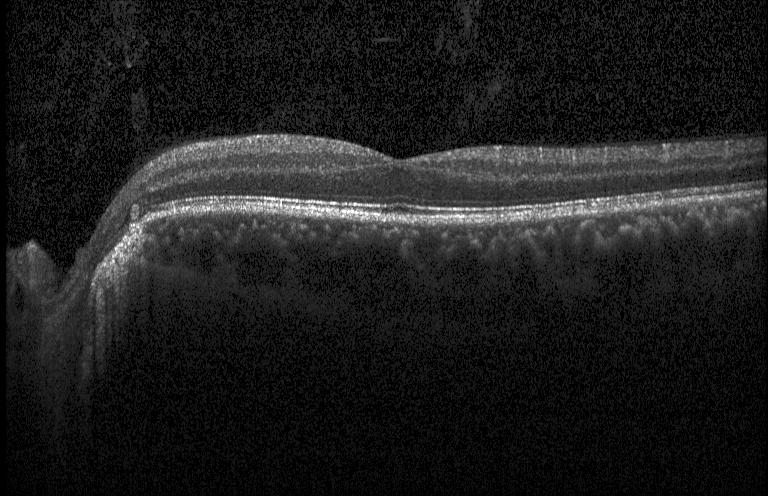
Horizontal scan through the fovea, OCT line scan. Finding: neither choroidal neovascularization, diabetic macular edema, nor drusen.